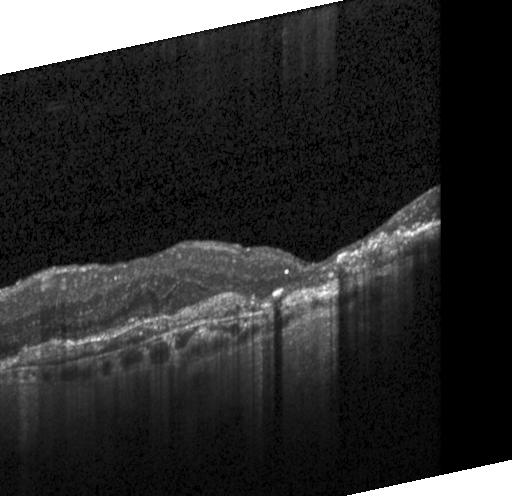
Fovea-centered; retinal OCT B-scan — A choroidal neovascular membrane.